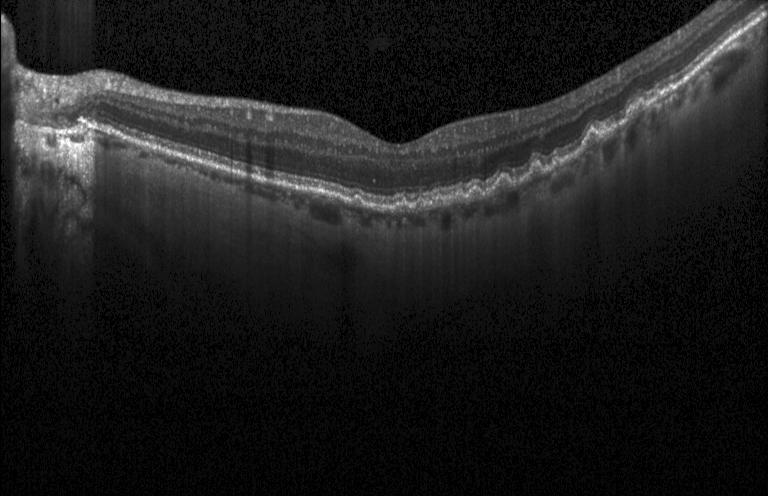
Assessment: sub-RPE drusenoid deposits.